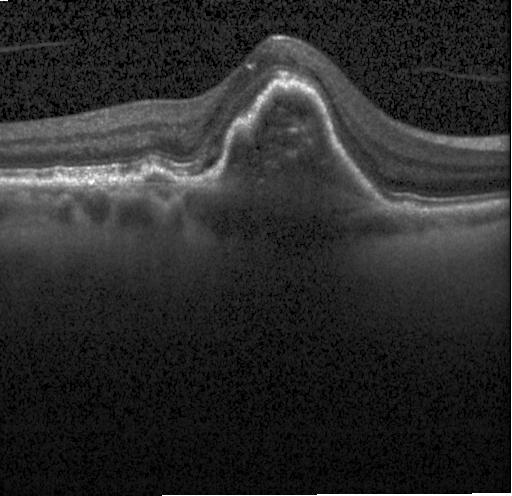

Heidelberg Spectralis OCT system, spectral-domain OCT, fovea-centered, retinal OCT B-scan — Dx: a choroidal neovascular membrane.